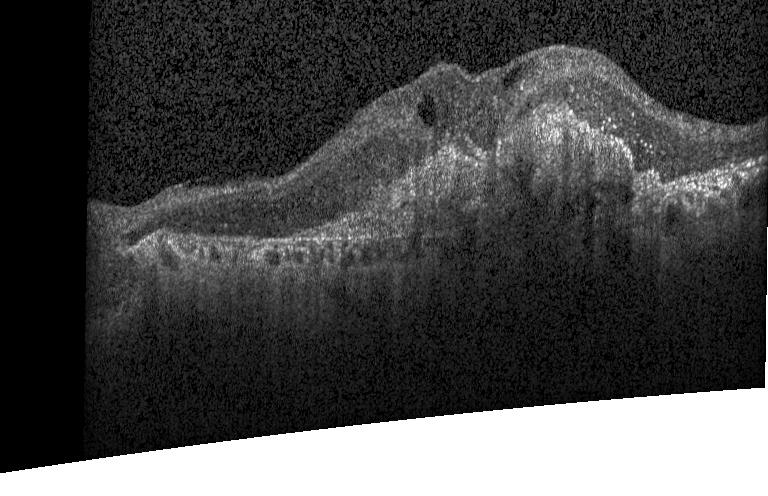

Fovea-centered; SD-OCT; Heidelberg Spectralis OCT system; OCT B-scan
CNV.